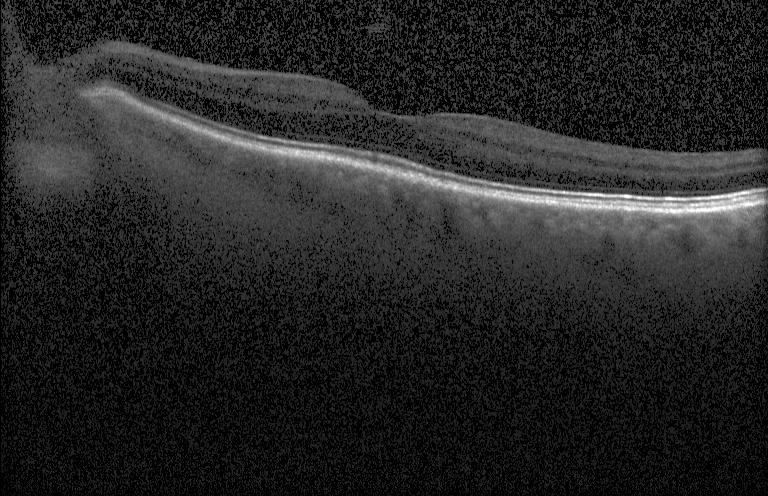 Retinal OCT cross-section showing no CNV, DME, or drusen.